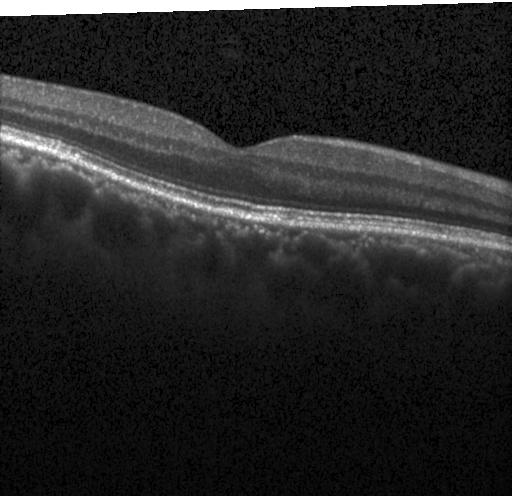 Dx: neither choroidal neovascularization, diabetic macular edema, nor drusen.